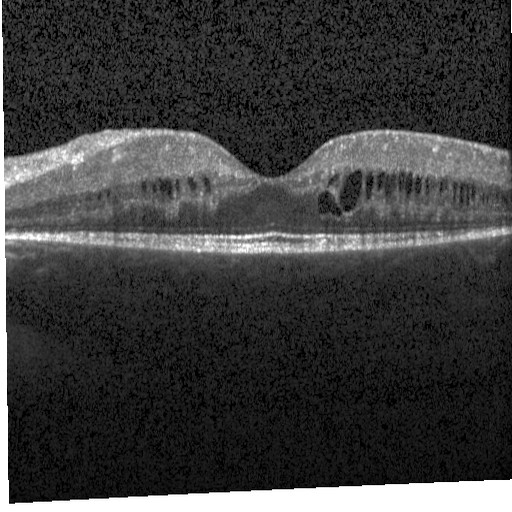 Optical coherence tomography B-scan · centered on the fovea · spectral-domain optical coherence tomography. The scan shows diabetic macular edema.